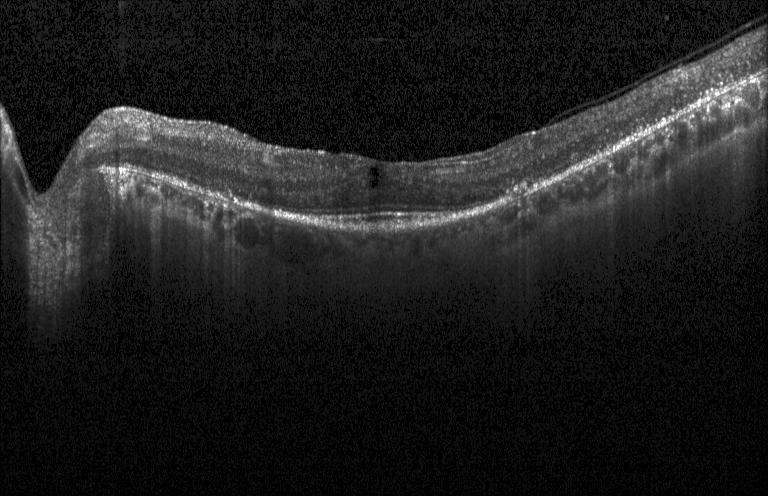 Macular OCT: DME.